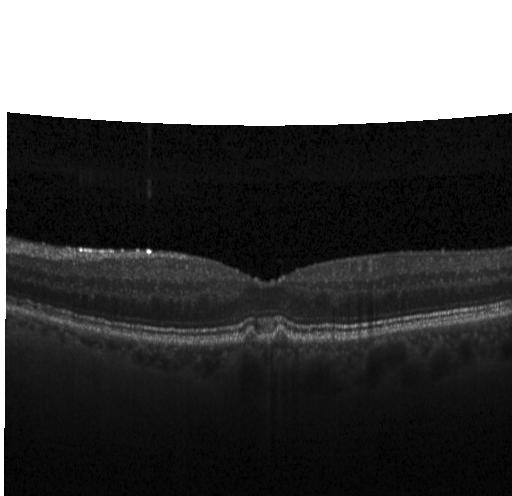

Assessment: sub-RPE drusenoid deposits.